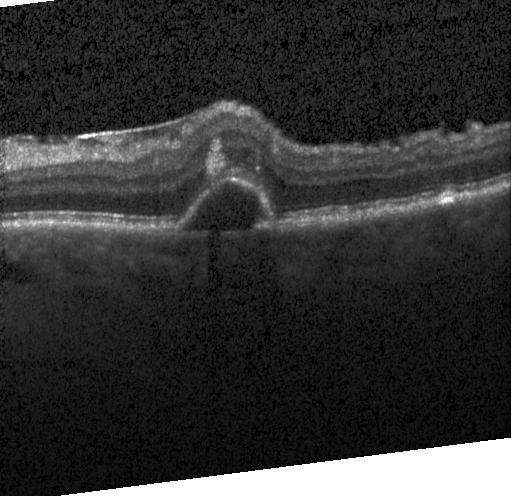 OCT scan showing CNV.